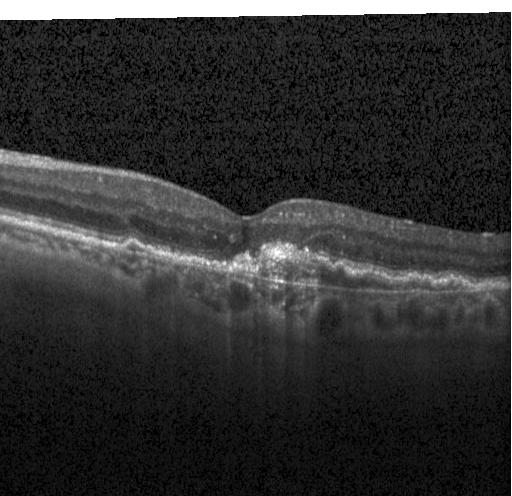
Finding: CNV.